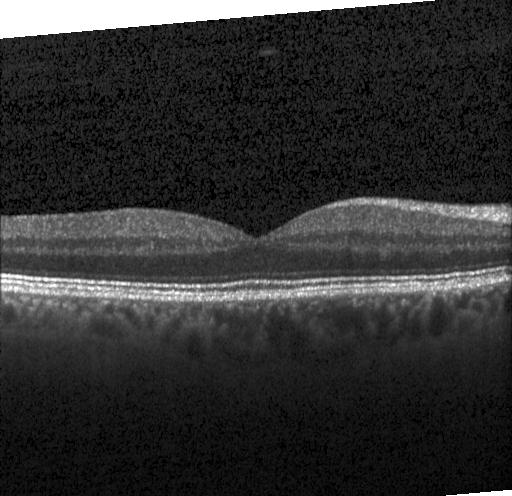
Retinal OCT B-scan — Diagnosis: no CNV, no DME, and no drusen.